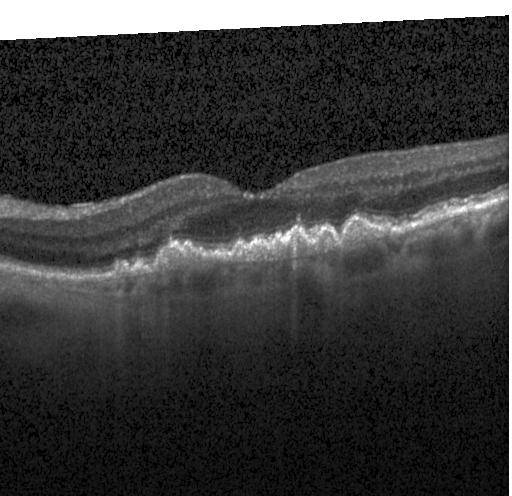

OCT finding: drusen.